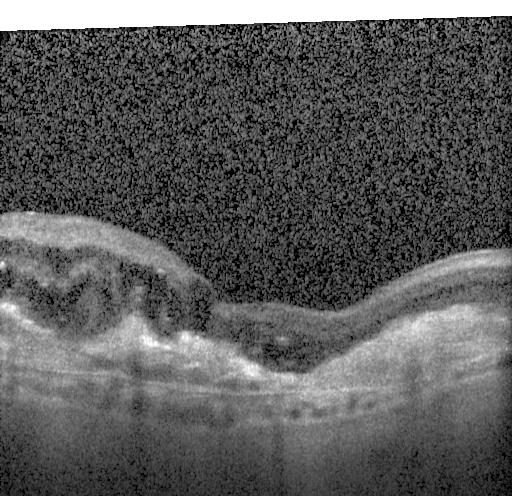
This B-scan demonstrates a choroidal neovascular membrane.